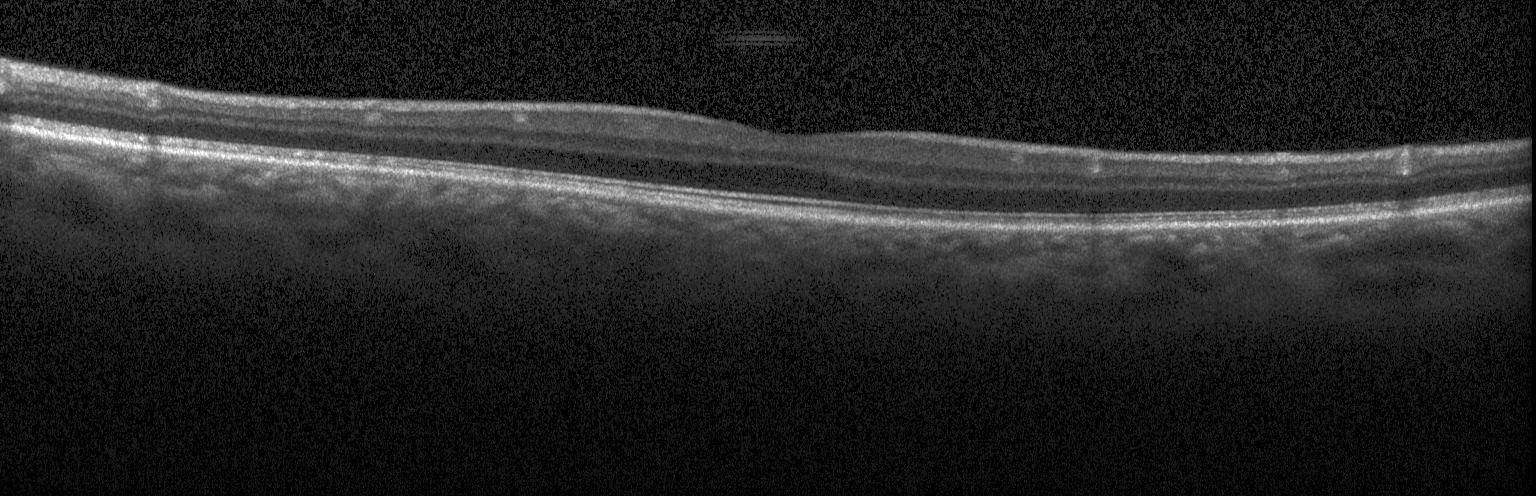

Macular OCT demonstrating no evidence of CNV, DME, or drusen.